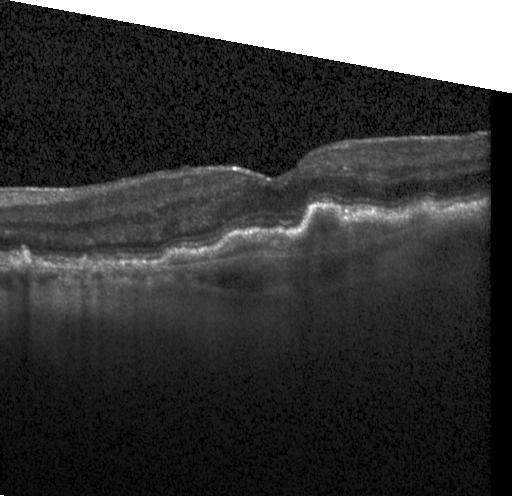
Spectral-domain OCT B-scan: a choroidal neovascular membrane.